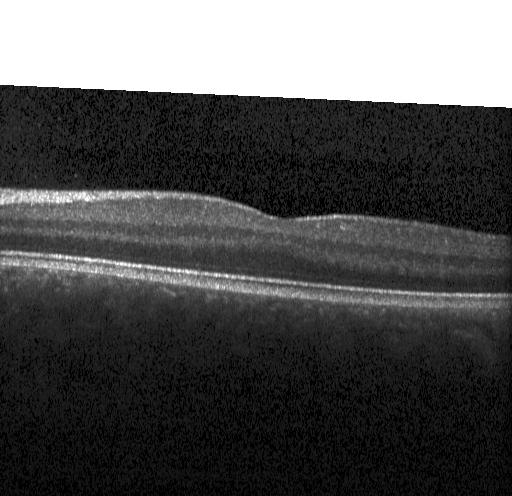
This B-scan demonstrates no evidence of choroidal neovascularization, diabetic macular edema, or drusen.